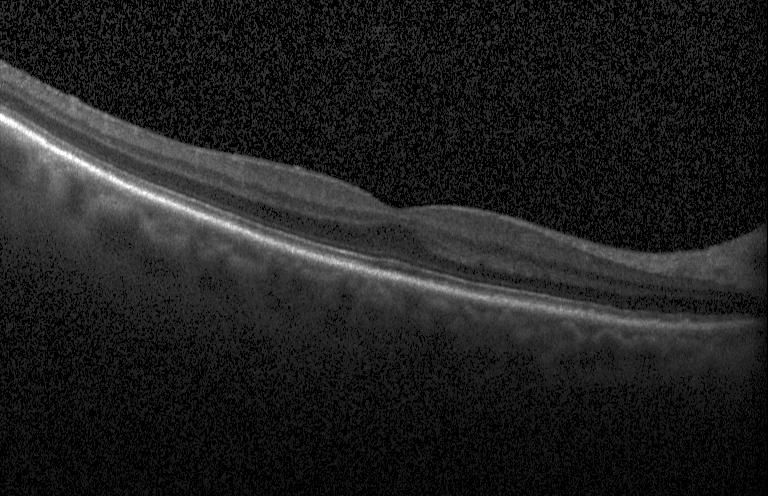

OCT B-scan showing no evidence of choroidal neovascularization, diabetic macular edema, or drusen.